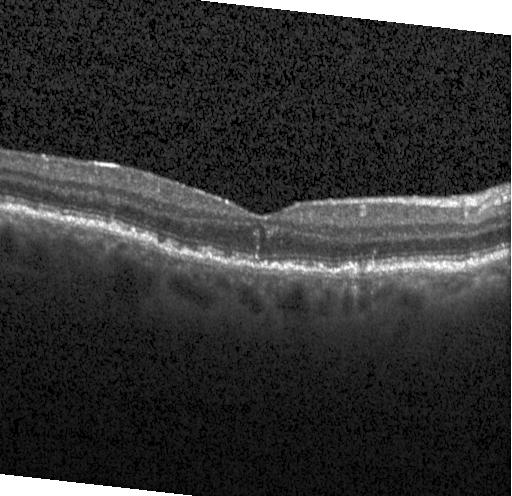

The scan shows multiple drusen.